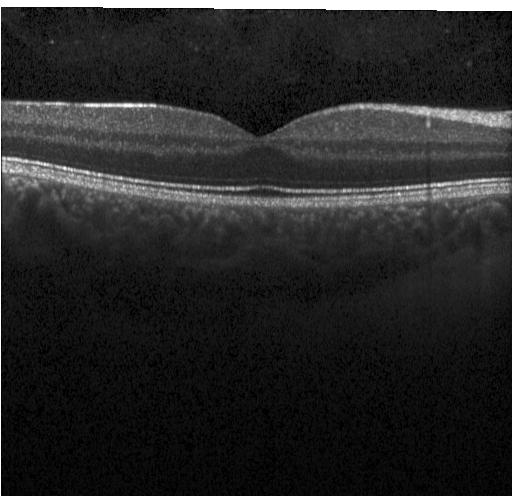

Macular scan · acquired on a Heidelberg Spectralis · OCT B-scan · spectral-domain optical coherence tomography.
Assessment: no evidence of choroidal neovascularization, diabetic macular edema, or drusen.